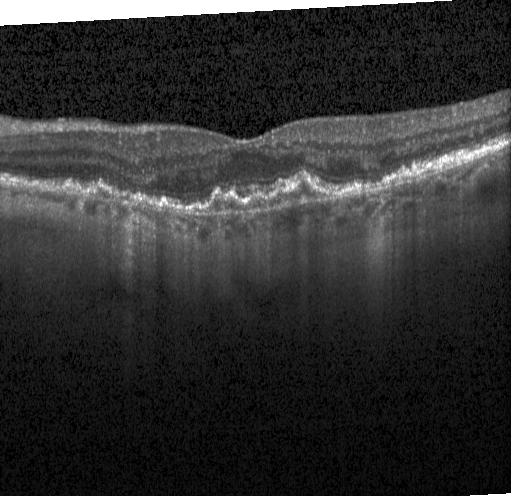 Instrument: Heidelberg Spectralis. Fovea-centered. Retinal OCT cross-section. SD-OCT
OCT finding: choroidal neovascularization.